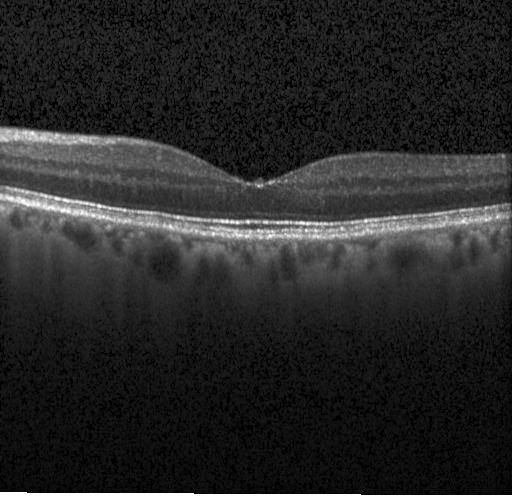
Macular OCT: no choroidal neovascularization, no diabetic macular edema, and no drusen.